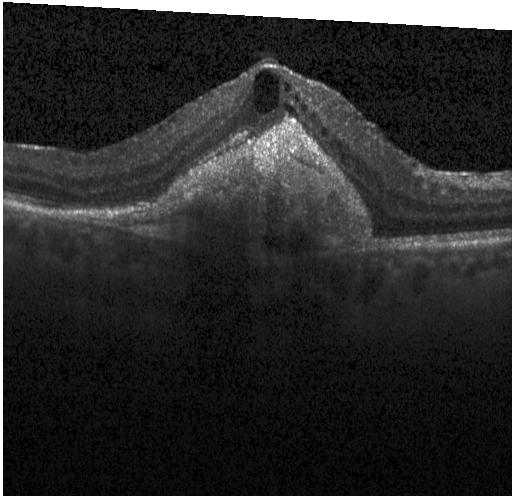
Dx: a choroidal neovascular membrane.